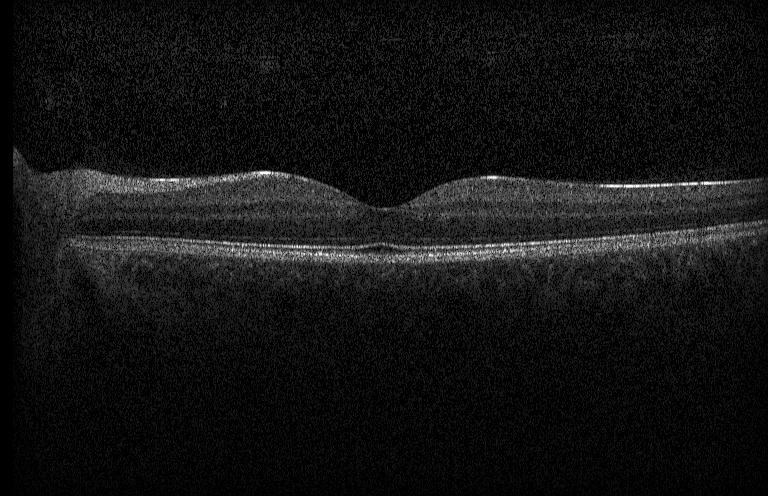

Spectral-domain OCT, acquired on a Heidelberg Spectralis, through the macula, optical coherence tomography scan. The scan shows no CNV, no DME, and no drusen.